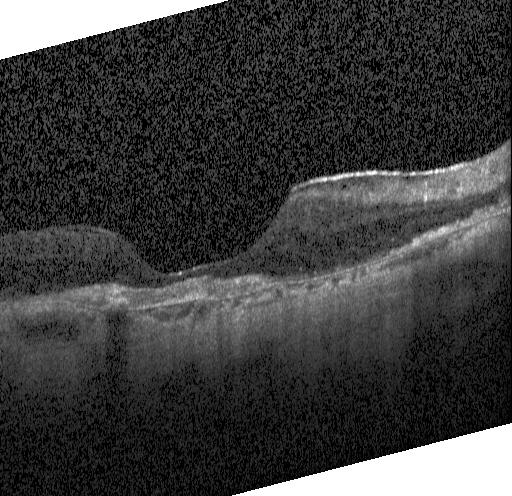 Spectral-domain OCT; through the macula; OCT B-scan
Impression: a choroidal neovascular membrane.